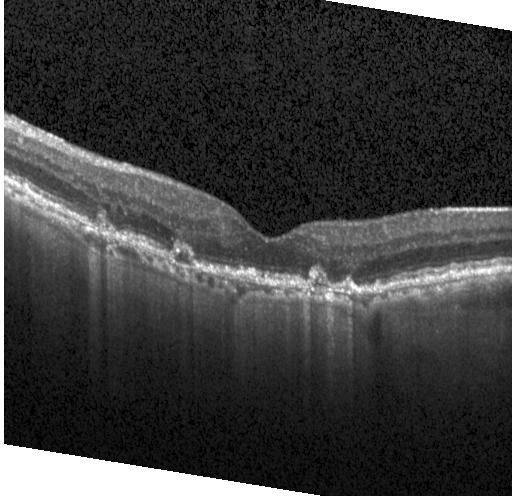

Optical coherence tomography scan.
The scan shows a choroidal neovascular membrane.